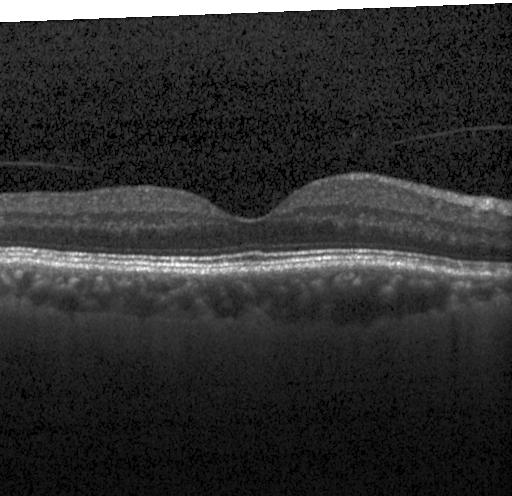

Macular OCT: no choroidal neovascularization, diabetic macular edema, or drusen.